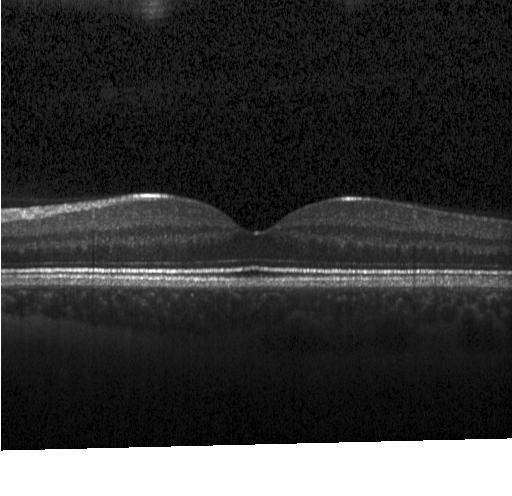

Retinal OCT B-scan. Spectral-domain optical coherence tomography. Through the macula
OCT finding: neither choroidal neovascularization, diabetic macular edema, nor drusen.